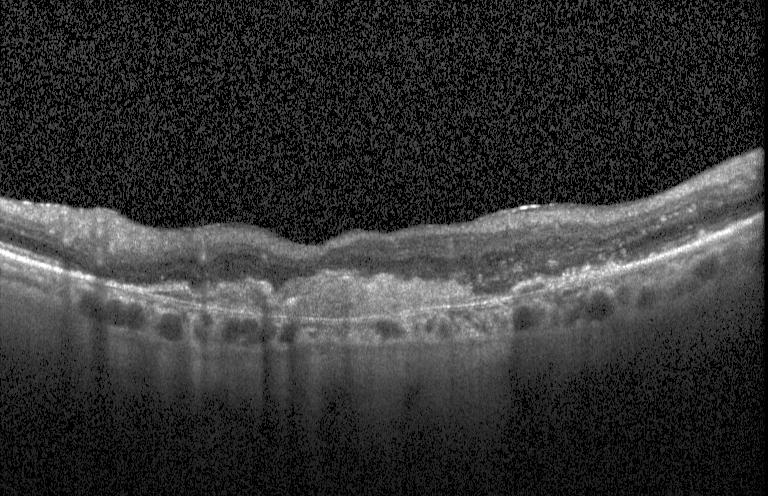 OCT finding: a choroidal neovascular membrane.